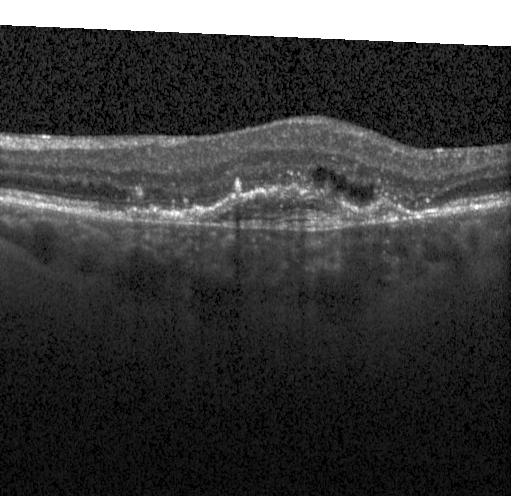

OCT B-scan; spectral-domain OCT; through the macula. The scan shows a choroidal neovascular membrane.